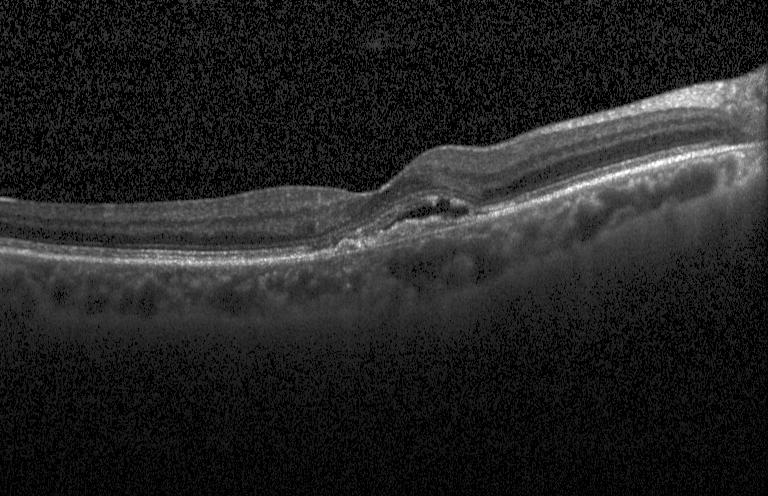 OCT line scan — CNV.